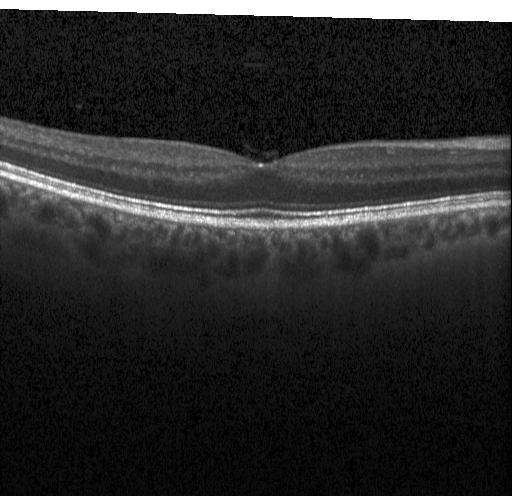
Instrument: Heidelberg Spectralis; spectral-domain optical coherence tomography; through the macula; optical coherence tomography scan — Finding: no choroidal neovascularization, no diabetic macular edema, and no drusen.